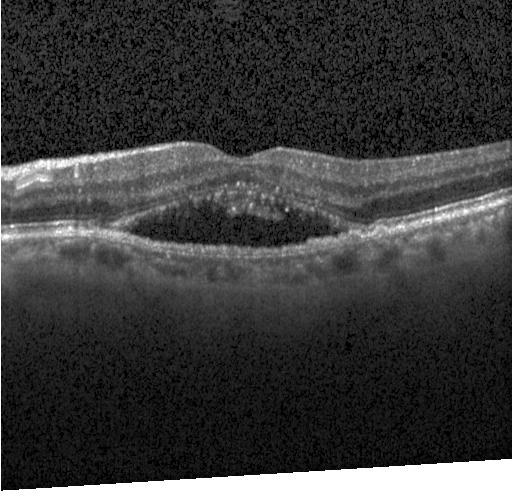
Spectral-domain OCT · OCT B-scan · Heidelberg Spectralis OCT system
The scan shows CNV.